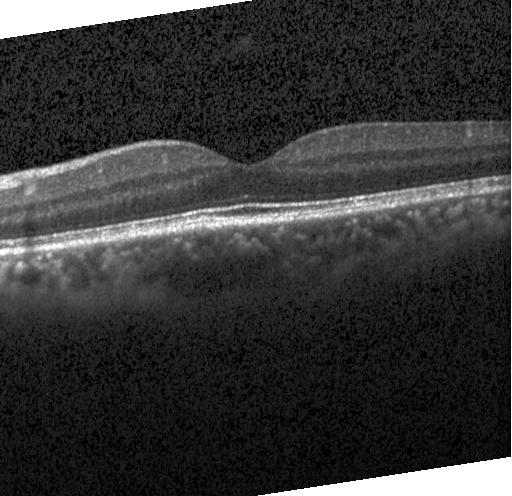 Assessment: neither choroidal neovascularization, diabetic macular edema, nor drusen.